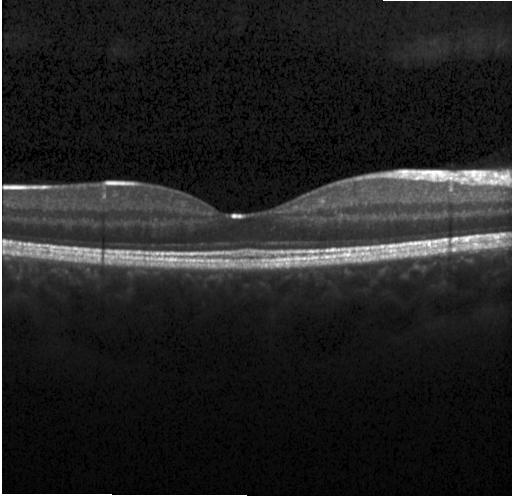

Retinal OCT cross-section showing no choroidal neovascularization, diabetic macular edema, or drusen.